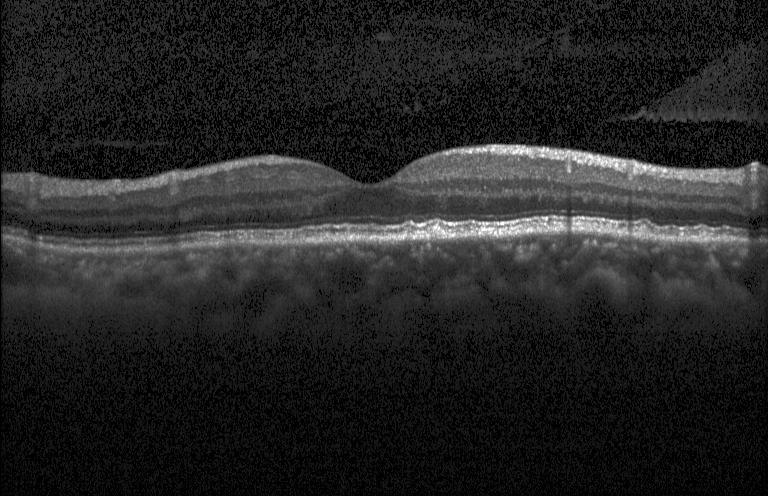 Optical coherence tomography scan.
This B-scan demonstrates sub-RPE drusenoid deposits.